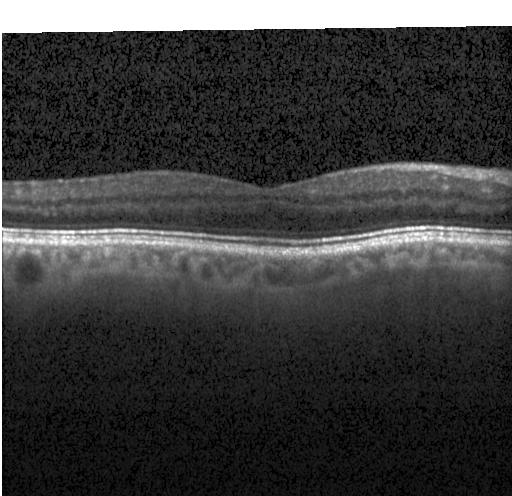 Assessment: no choroidal neovascularization, no diabetic macular edema, and no drusen.